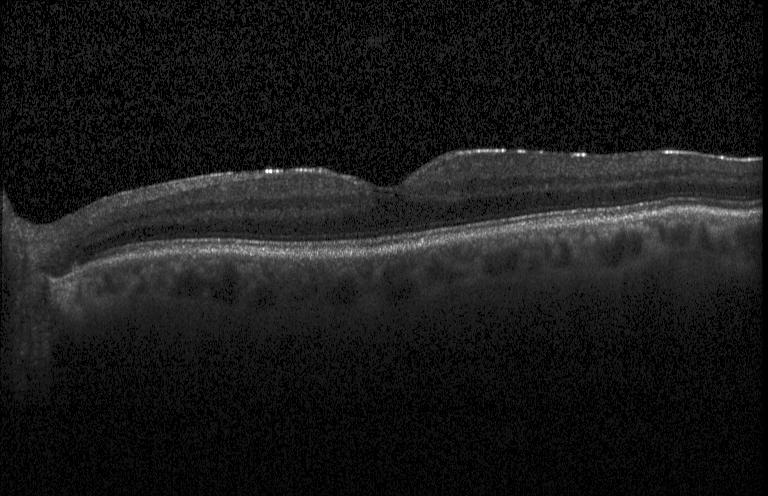

Spectral-domain OCT. OCT B-scan
Macular OCT: no choroidal neovascularization, diabetic macular edema, or drusen.